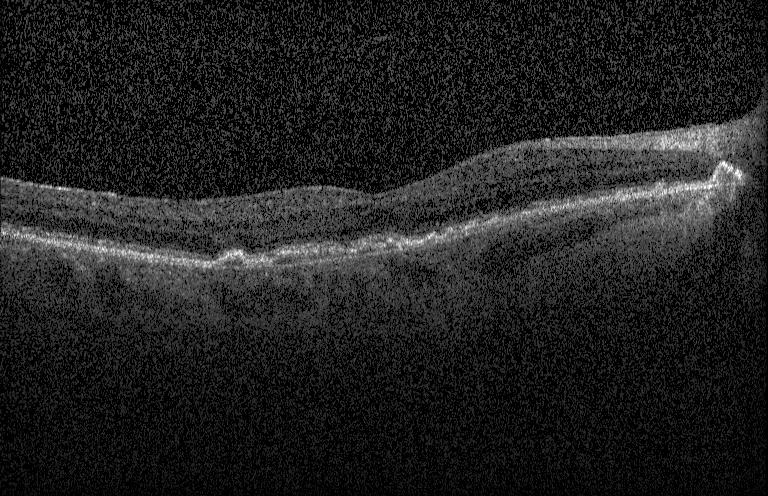
A choroidal neovascular membrane.